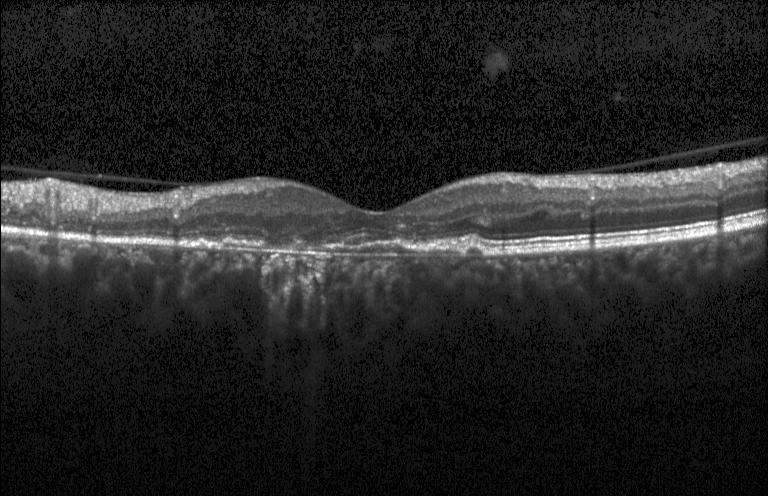

Macular scan; spectral-domain optical coherence tomography; optical coherence tomography scan.
Finding: choroidal neovascularization (CNV).